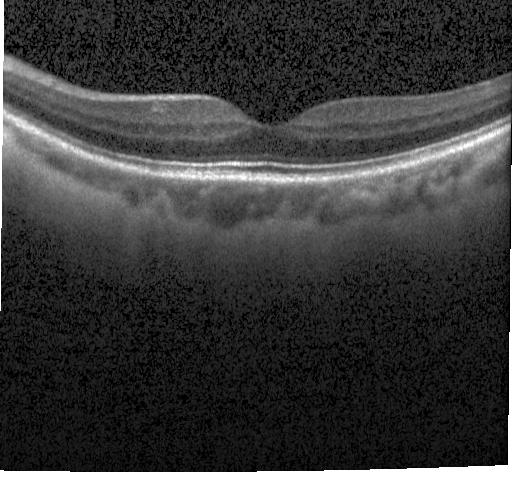 OCT B-scan showing no CNV, no DME, and no drusen.